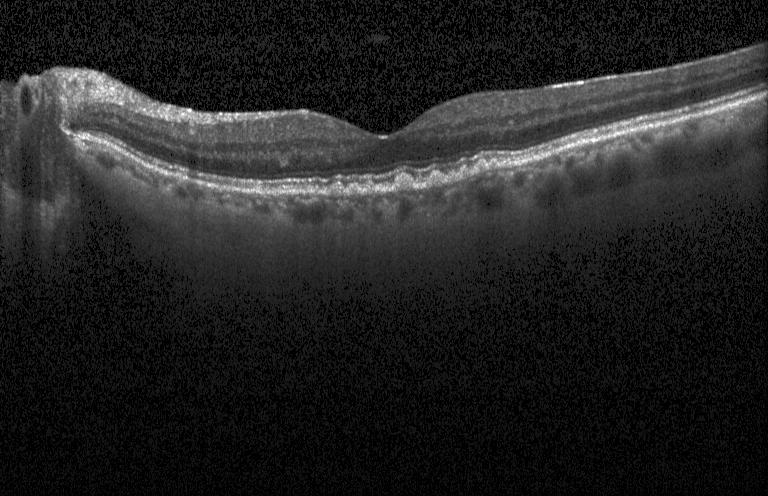 Retinal OCT B-scan
Finding: drusen.